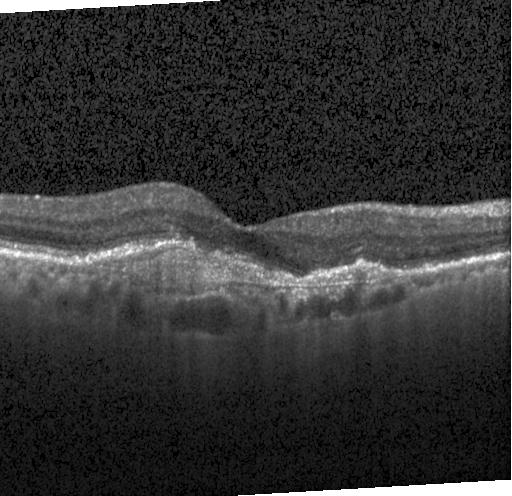
Optical coherence tomography scan; SD-OCT — This B-scan demonstrates a choroidal neovascular membrane.